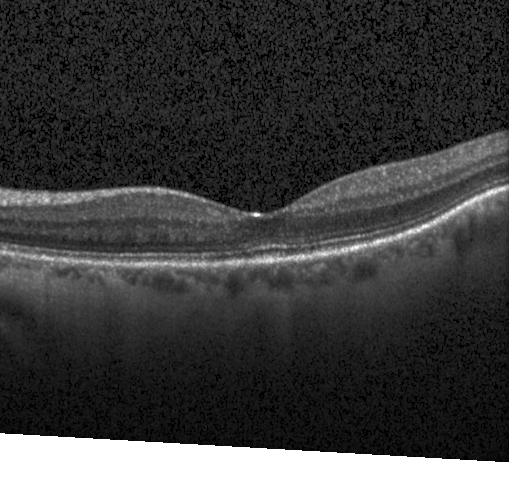
Macular OCT: no choroidal neovascularization, no diabetic macular edema, and no drusen.